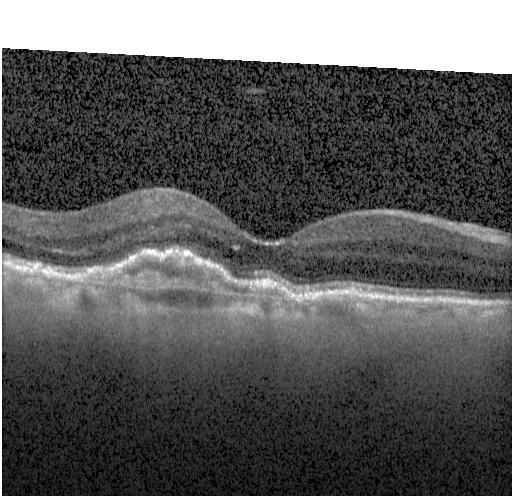

Optical coherence tomography B-scan.
The scan shows choroidal neovascularization.